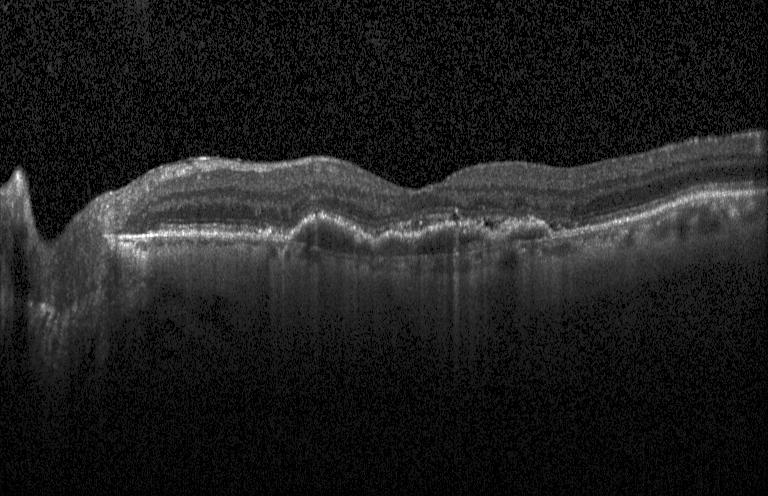 SD-OCT · OCT B-scan · Heidelberg Spectralis — The scan shows a choroidal neovascular membrane.